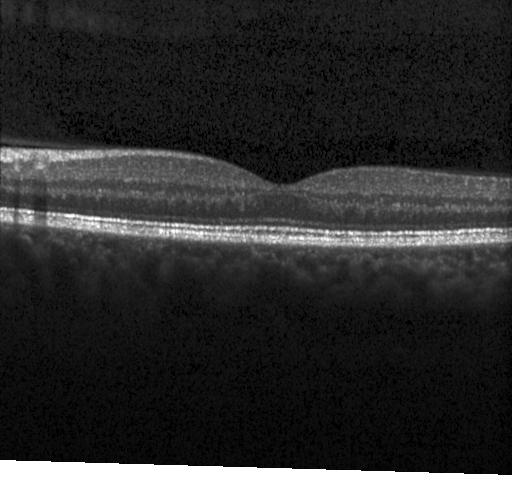

Spectral-domain OCT. Horizontal scan through the fovea. OCT line scan — OCT finding: no CNV, DME, or drusen.